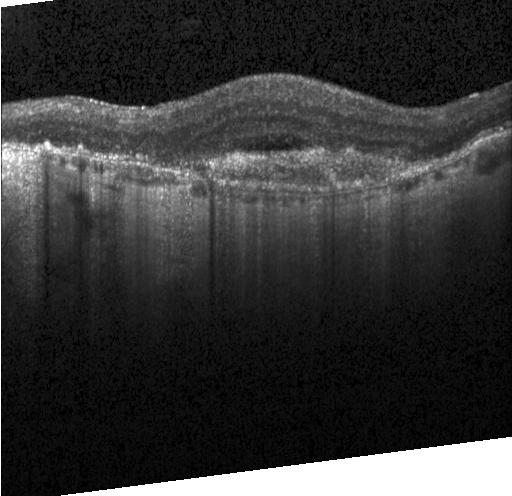
Optical coherence tomography scan.
Finding: CNV.